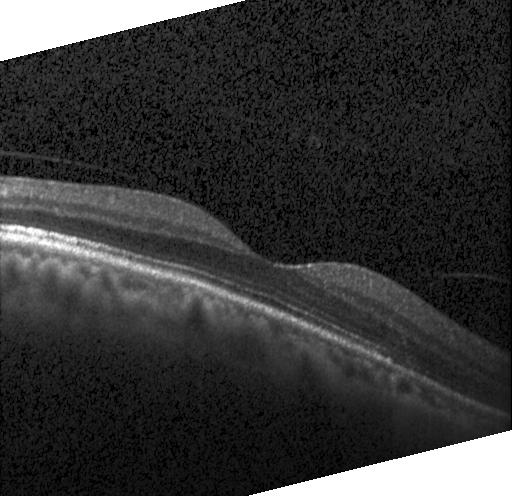

Diagnosis: no choroidal neovascularization, no diabetic macular edema, and no drusen.